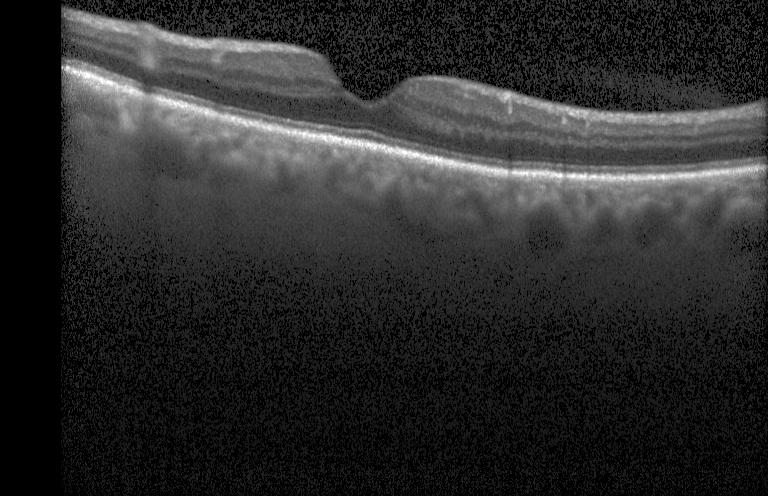
Finding: no evidence of choroidal neovascularization, diabetic macular edema, or drusen.